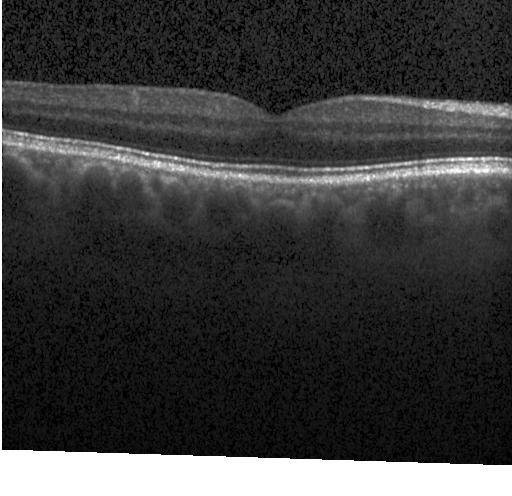 Optical coherence tomography B-scan. Horizontal scan through the fovea.
This B-scan demonstrates no choroidal neovascularization, no diabetic macular edema, and no drusen.